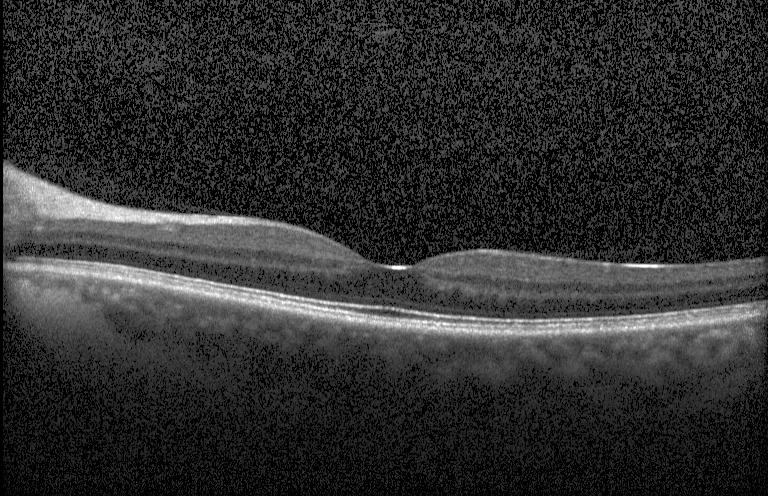
Through the macula, SD-OCT, OCT line scan, Heidelberg Spectralis OCT system
Dx: no evidence of choroidal neovascularization, diabetic macular edema, or drusen.